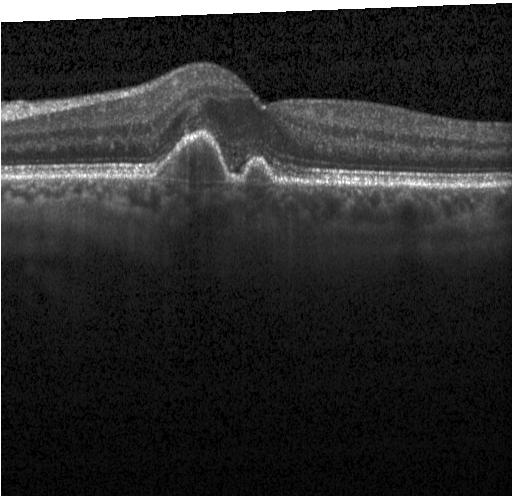 Spectral-domain OCT B-scan: a choroidal neovascular membrane.